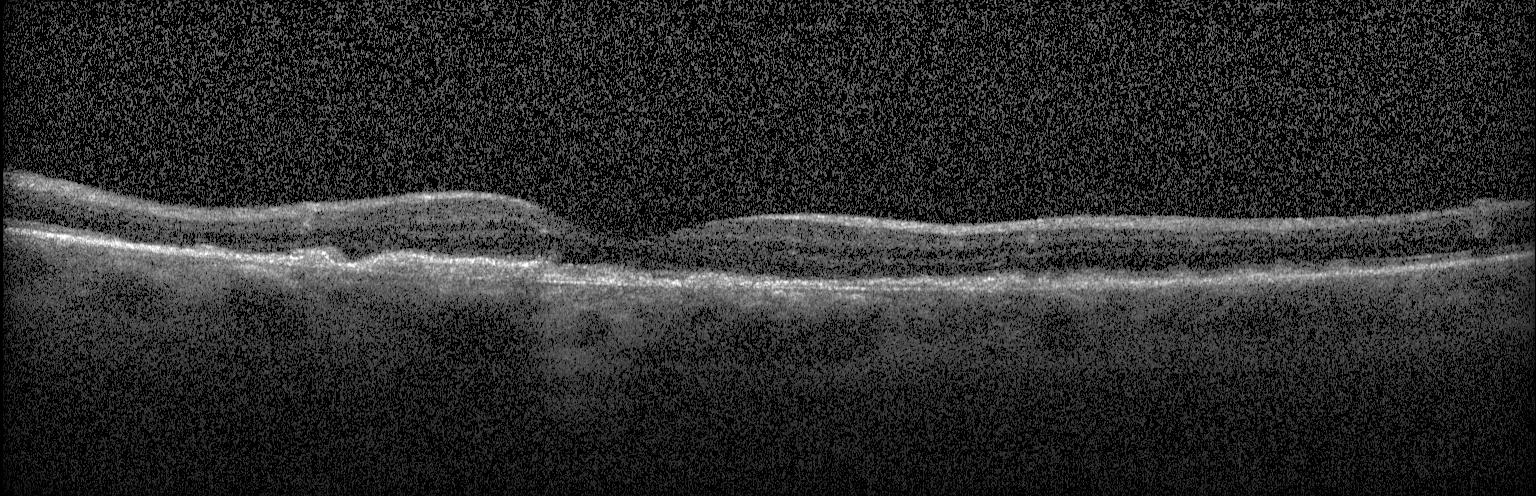 Heidelberg Spectralis OCT system; horizontal scan through the fovea; spectral-domain OCT; retinal OCT B-scan — Finding: a choroidal neovascular membrane.